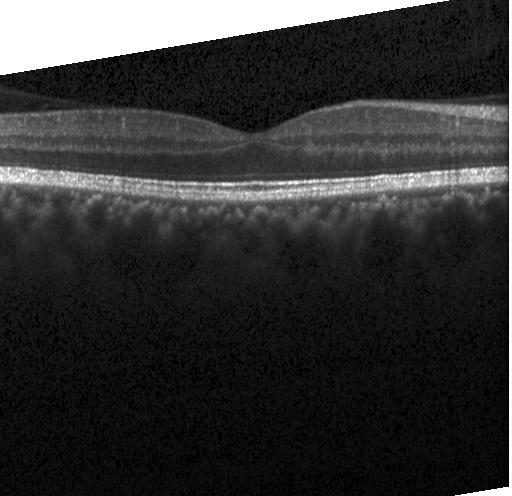 Instrument: Heidelberg Spectralis · OCT line scan · horizontal scan through the fovea · spectral-domain OCT
Macular OCT: no choroidal neovascularization, diabetic macular edema, or drusen.